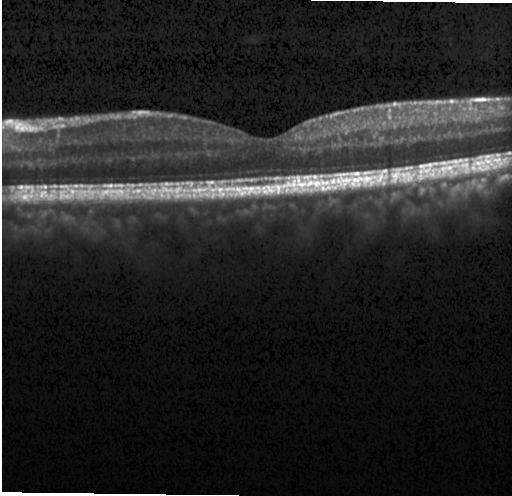

Retinal OCT B-scan; Heidelberg Spectralis; spectral-domain OCT; macular scan
Finding: neither choroidal neovascularization, diabetic macular edema, nor drusen.